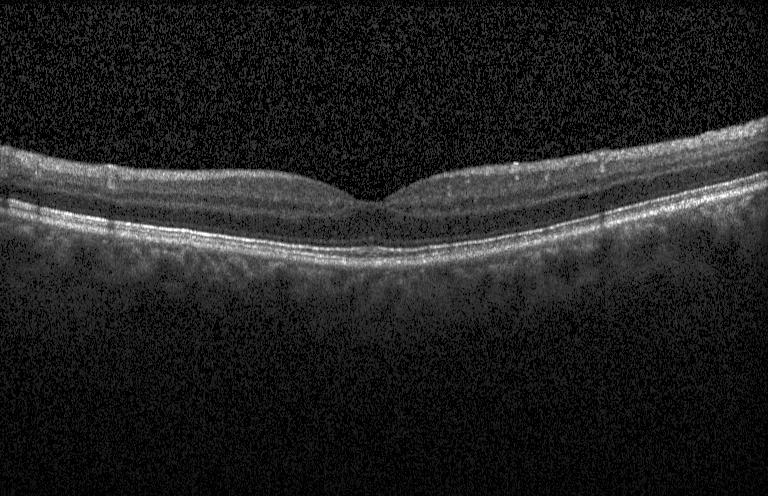

This B-scan demonstrates neither choroidal neovascularization, diabetic macular edema, nor drusen.